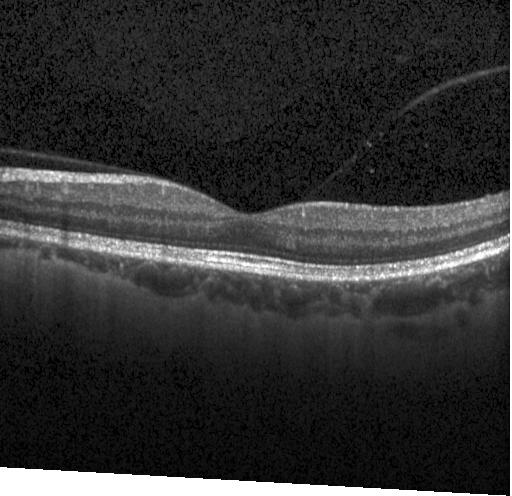 Optical coherence tomography scan
Assessment: no choroidal neovascularization, diabetic macular edema, or drusen.